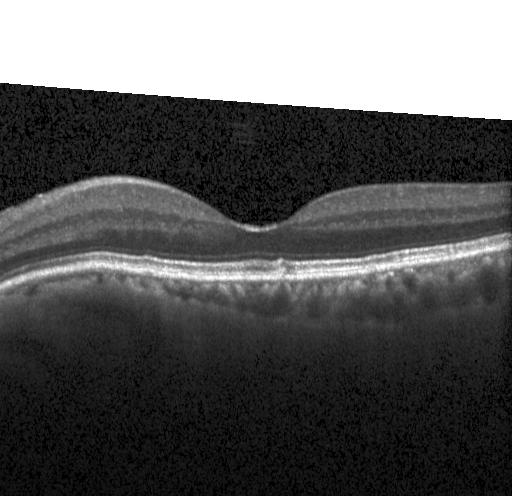
Spectral-domain OCT; retinal OCT cross-section; macular scan.
Diagnosis: multiple drusen.